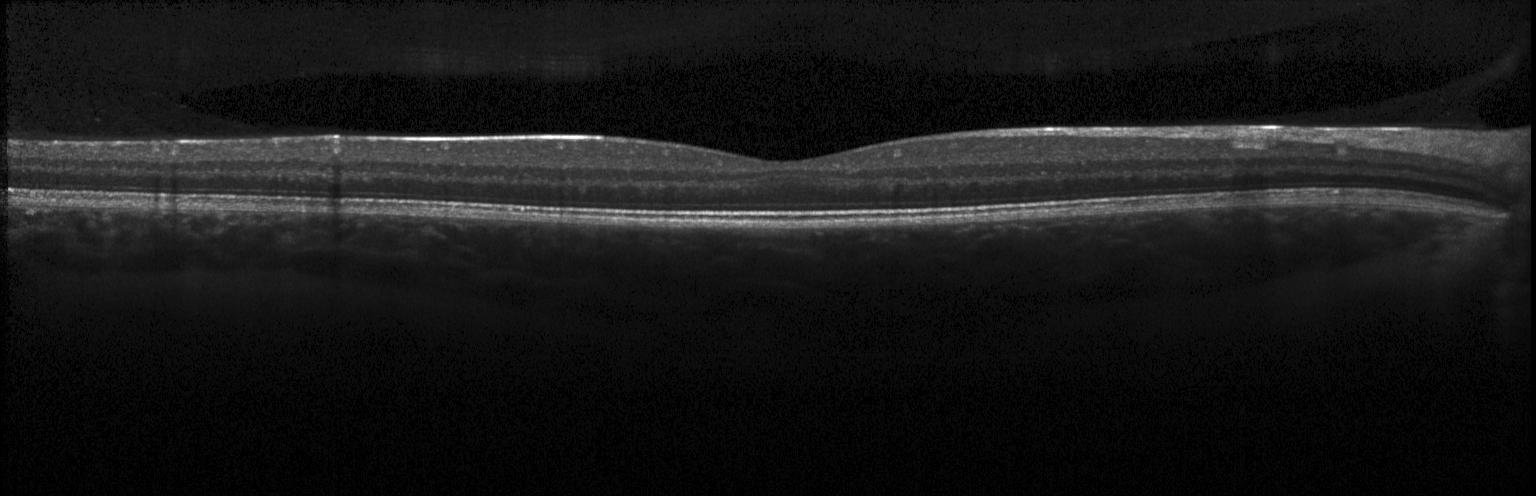

Heidelberg Spectralis OCT system; optical coherence tomography B-scan.
No choroidal neovascularization, no diabetic macular edema, and no drusen.